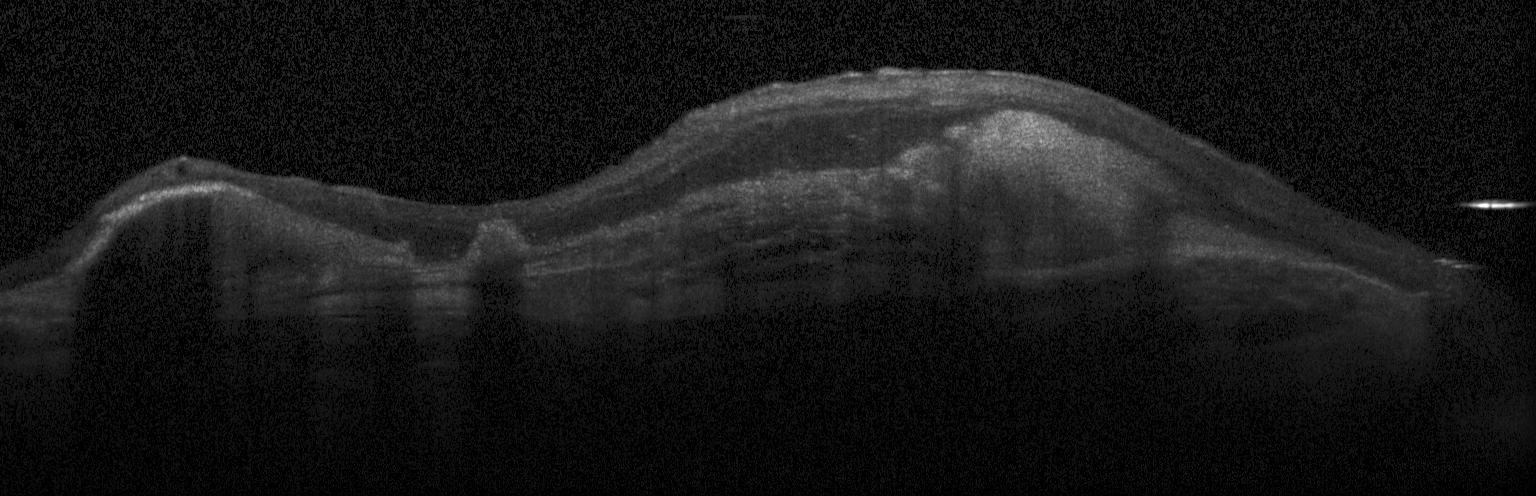 Diagnosis: a choroidal neovascular membrane.